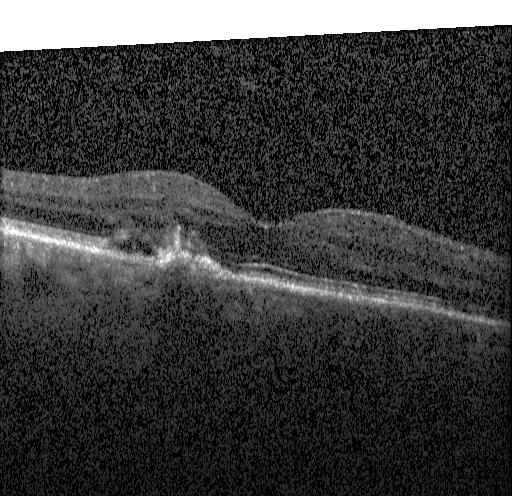
OCT B-scan
OCT finding: choroidal neovascularization (CNV).